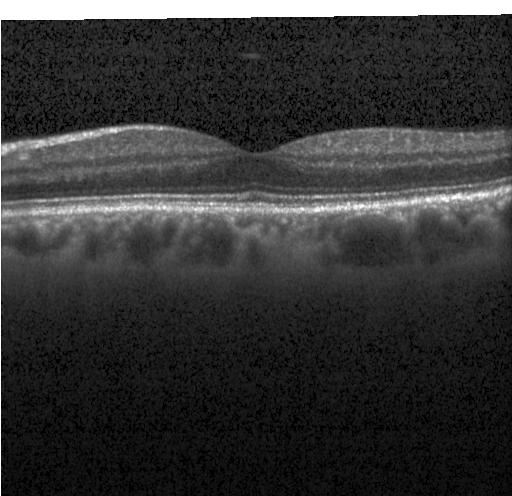

SD-OCT · Heidelberg Spectralis · OCT B-scan
OCT finding: no choroidal neovascularization, diabetic macular edema, or drusen.